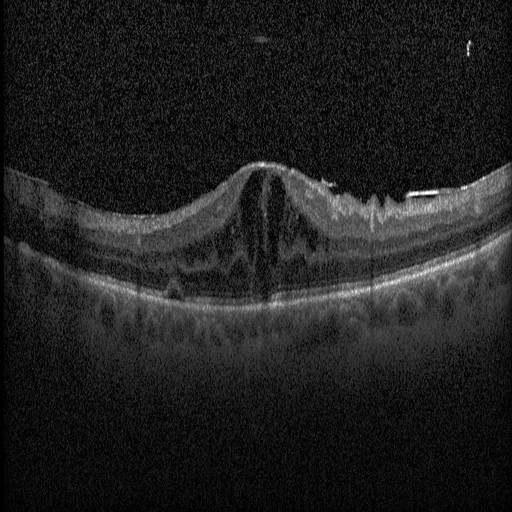 Fovea-centered · spectral-domain optical coherence tomography · acquired on a Heidelberg Spectralis · retinal OCT cross-section.
Finding: diabetic macular edema.